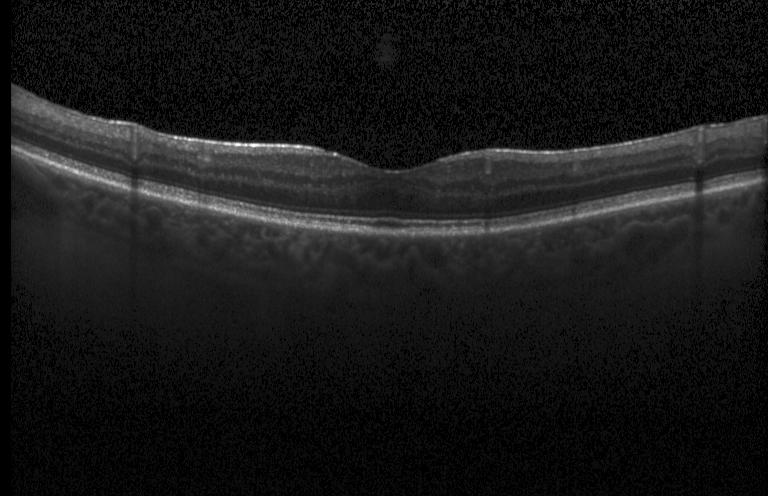 Spectral-domain optical coherence tomography · centered on the fovea · Heidelberg Spectralis OCT system · OCT B-scan — The scan shows no choroidal neovascularization, no diabetic macular edema, and no drusen.